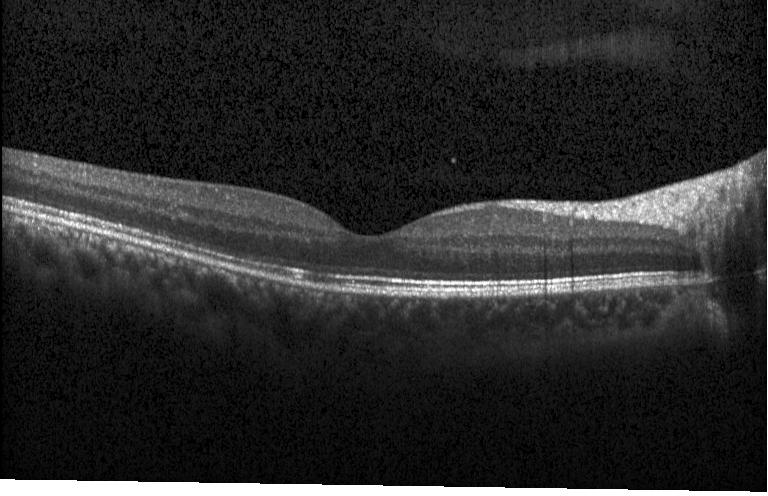

Centered on the fovea; OCT B-scan. This B-scan demonstrates no CNV, no DME, and no drusen.